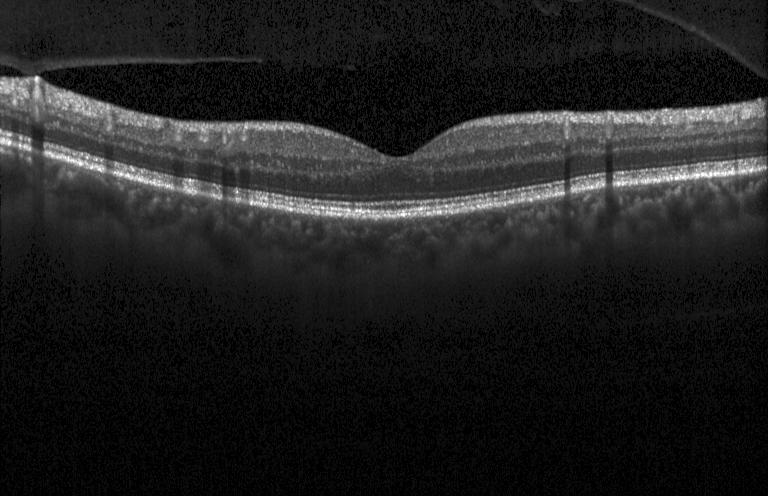 Finding: no choroidal neovascularization, diabetic macular edema, or drusen.